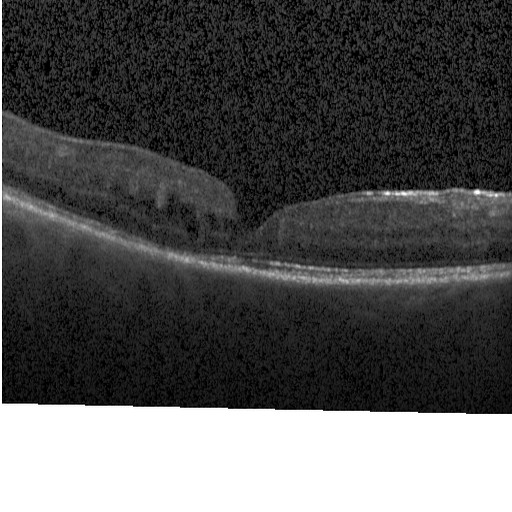 The scan shows diabetic macular edema.